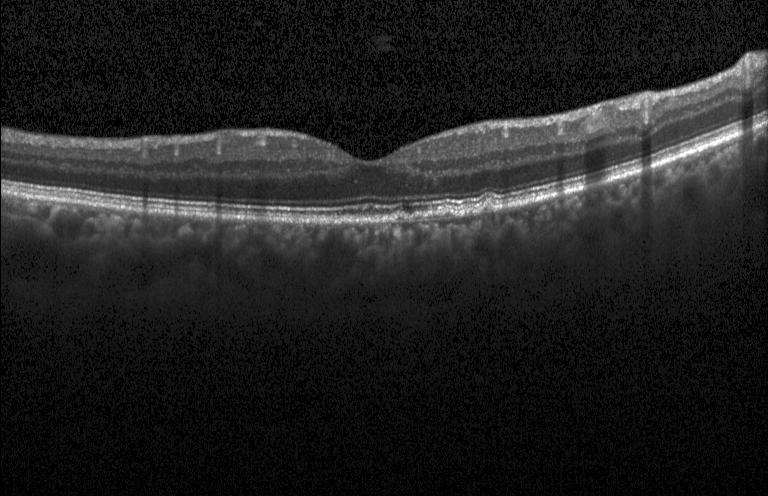 Retinal OCT cross-section showing drusen.